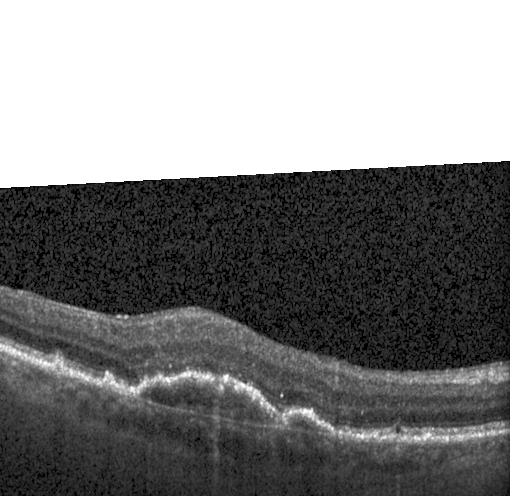

OCT line scan — OCT finding: choroidal neovascularization.